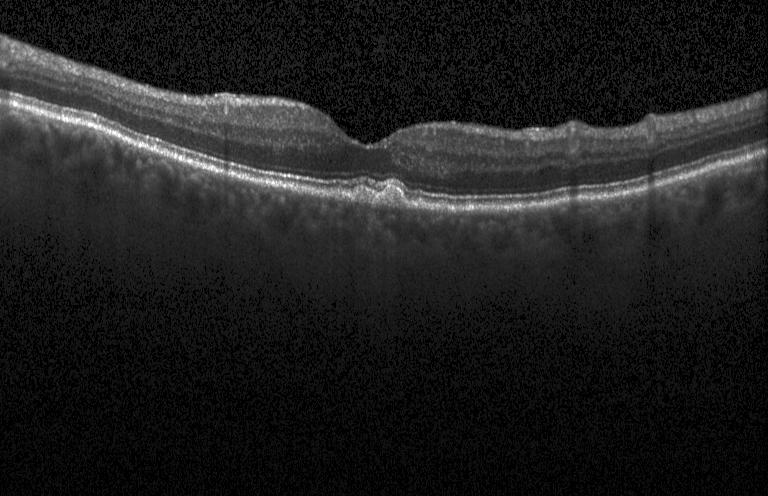

OCT B-scan. The scan shows multiple drusen.